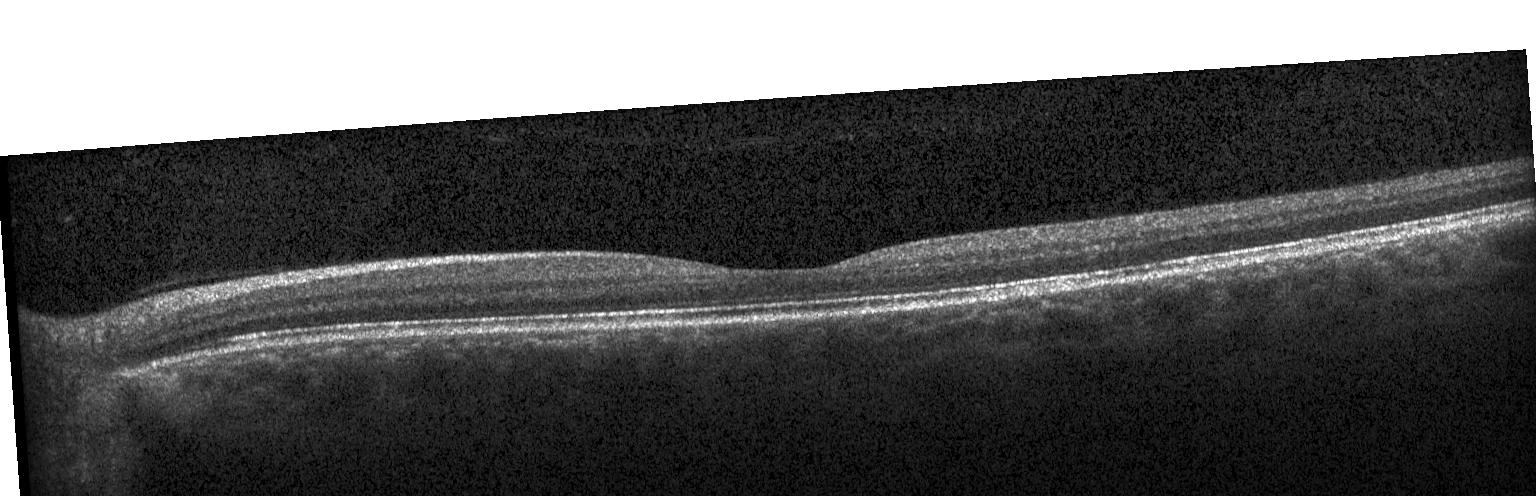

Heidelberg Spectralis; SD-OCT; optical coherence tomography scan; fovea-centered — Impression: neither CNV, DME, nor drusen.